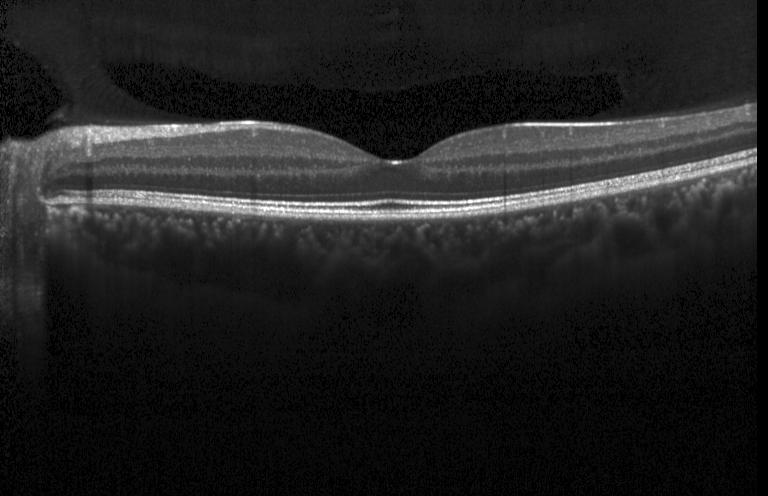

Retinal OCT B-scan · SD-OCT · Heidelberg Spectralis · through the macula. Dx: no choroidal neovascularization, no diabetic macular edema, and no drusen.